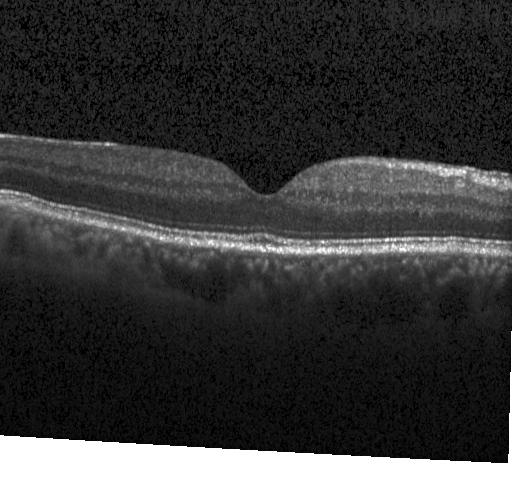

Macular OCT demonstrating no evidence of choroidal neovascularization, diabetic macular edema, or drusen.